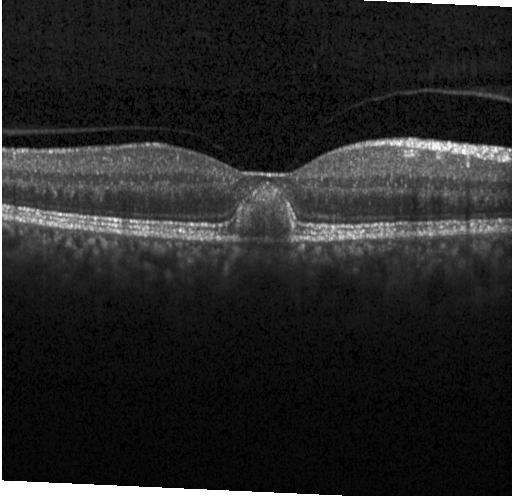
Finding: choroidal neovascularization.